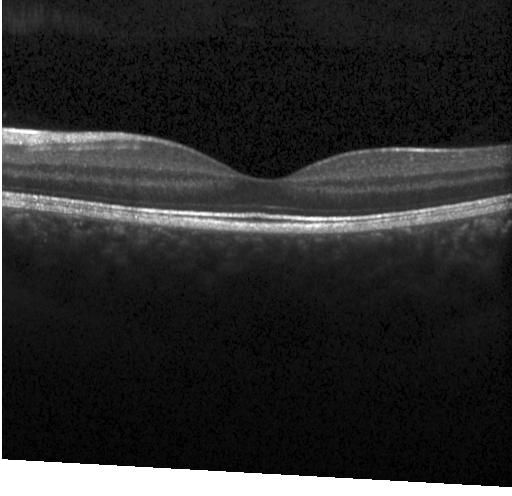

Spectral-domain OCT, optical coherence tomography scan, Heidelberg Spectralis
Finding: neither CNV, DME, nor drusen.